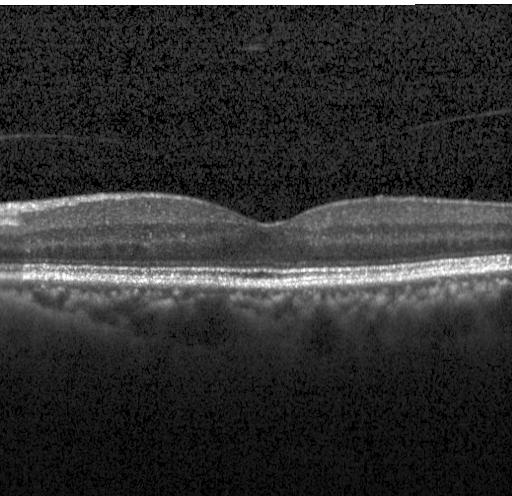

Retinal OCT cross-section showing no CNV, no DME, and no drusen.